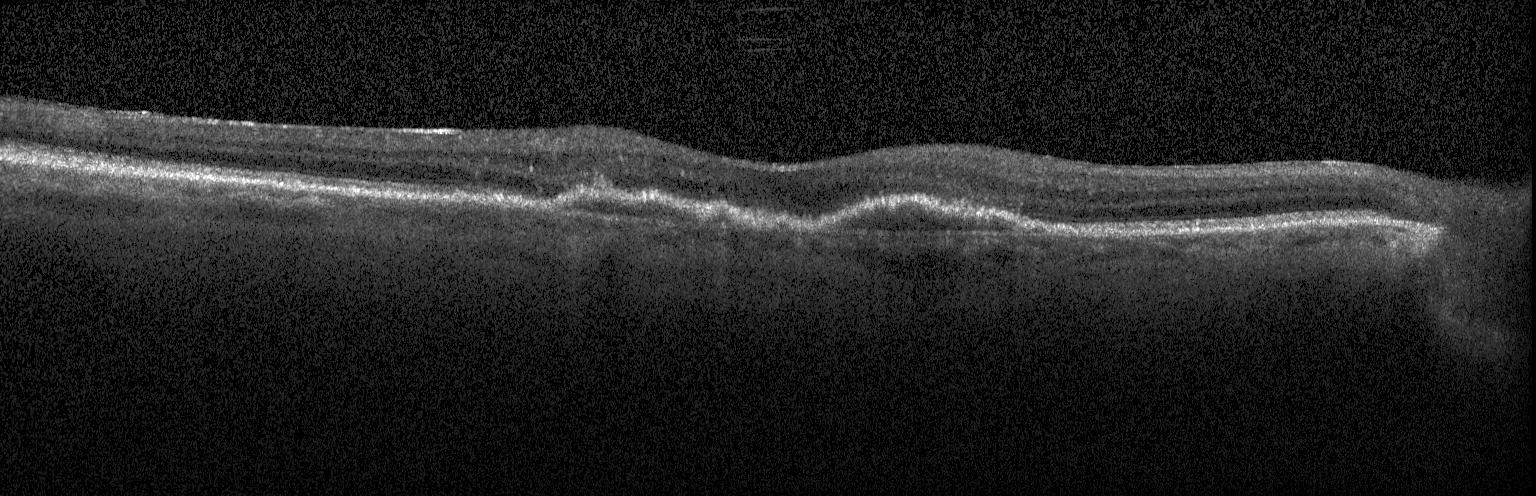
Horizontal scan through the fovea, Heidelberg Spectralis, spectral-domain OCT, OCT B-scan — This B-scan demonstrates a choroidal neovascular membrane.